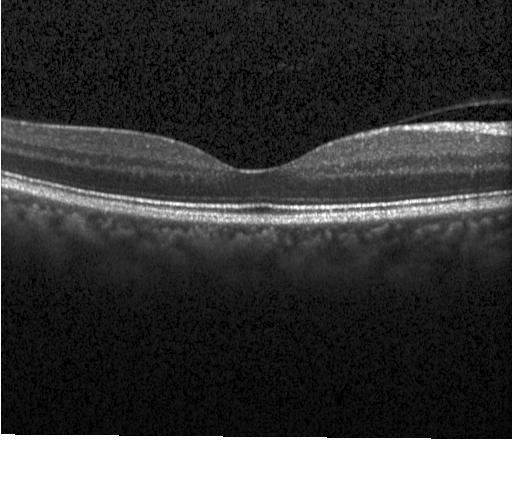
Macular OCT: no evidence of CNV, DME, or drusen.